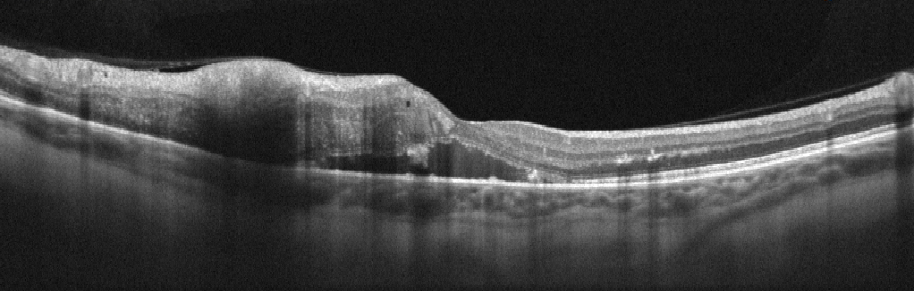

Optovue Avanti RTVue XR; OCT line scan — Impression: retinal vein occlusion (RVO).